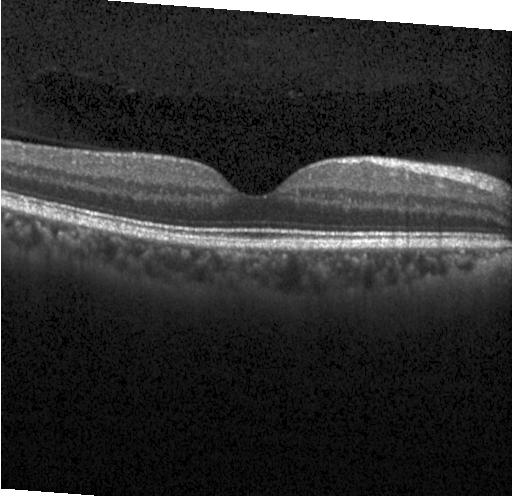
OCT line scan. Fovea-centered.
Macular OCT: no choroidal neovascularization, no diabetic macular edema, and no drusen.